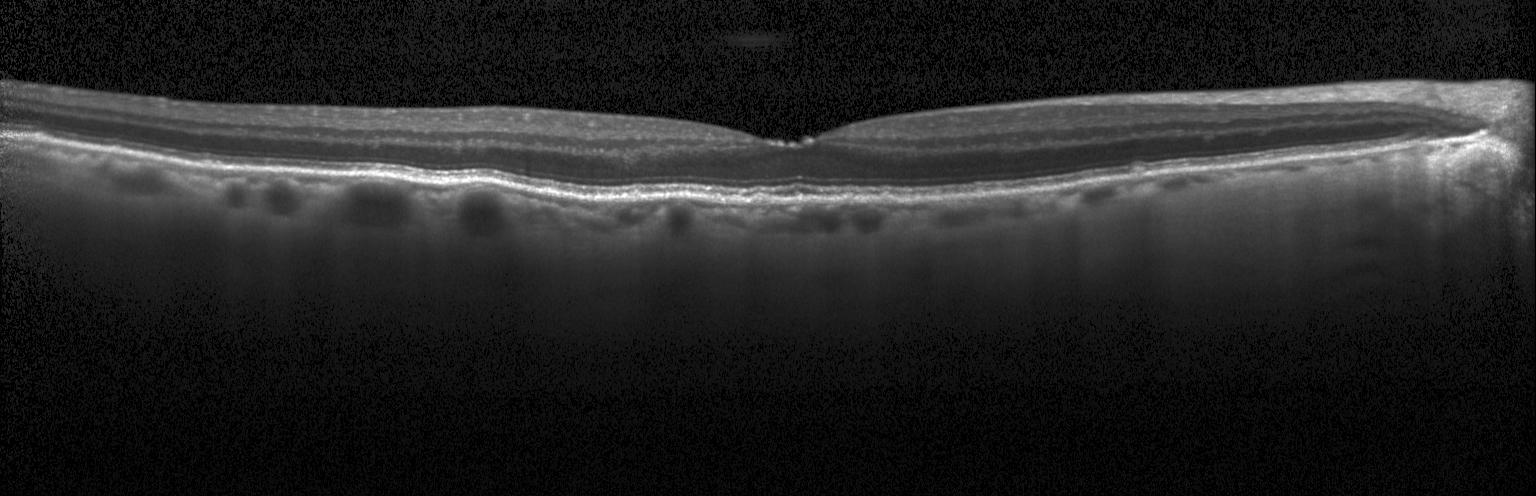

Optical coherence tomography scan. Through the macula. Impression: sub-RPE drusenoid deposits.